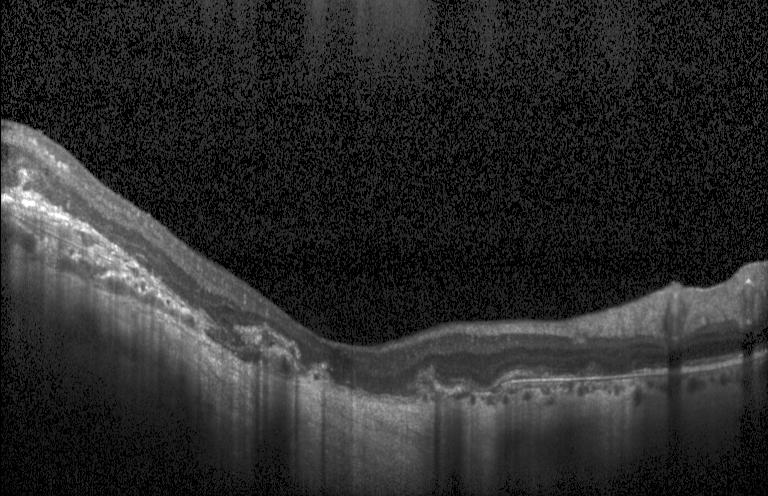

Finding: CNV.